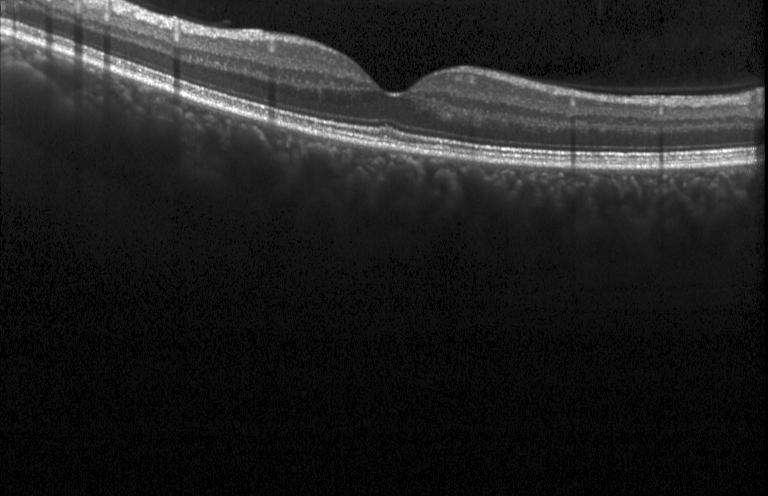

Spectral-domain optical coherence tomography. OCT B-scan. Centered on the fovea
The scan shows neither choroidal neovascularization, diabetic macular edema, nor drusen.